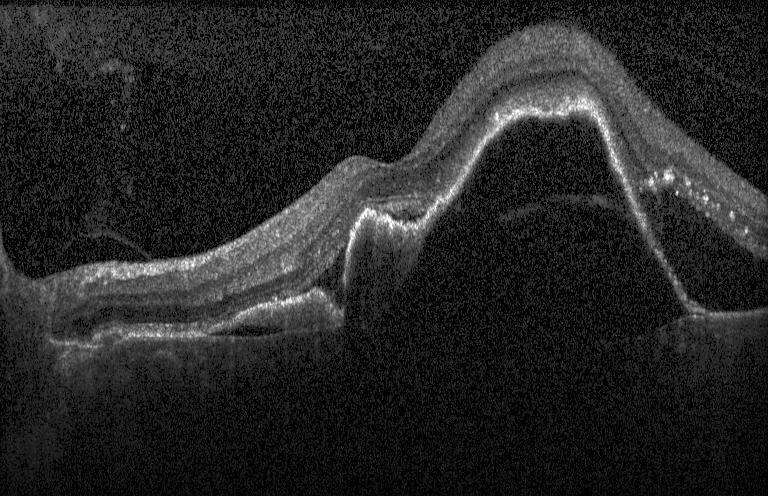
Retinal OCT B-scan · acquired on a Heidelberg Spectralis
Impression: a choroidal neovascular membrane.